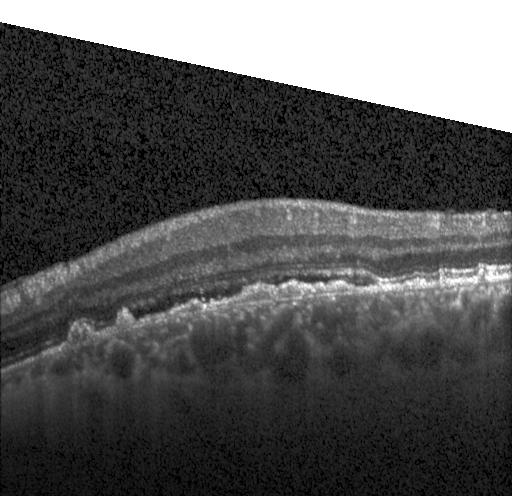
OCT line scan — Impression: choroidal neovascularization (CNV).